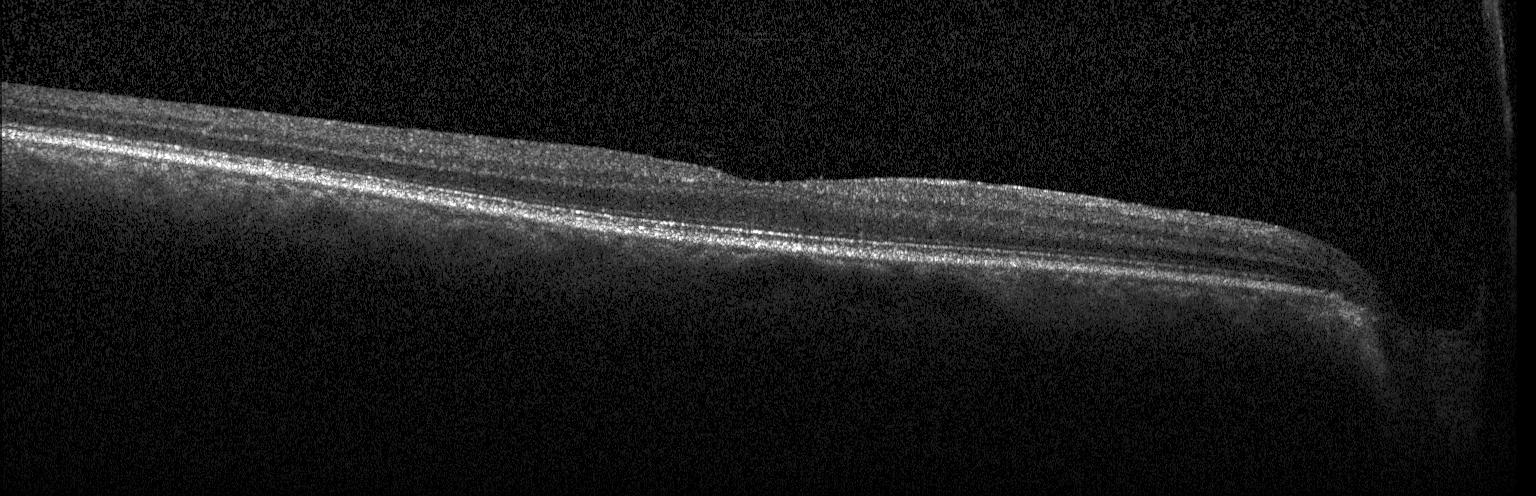

Optical coherence tomography scan · fovea-centered · Heidelberg Spectralis OCT system
Finding: no choroidal neovascularization, no diabetic macular edema, and no drusen.